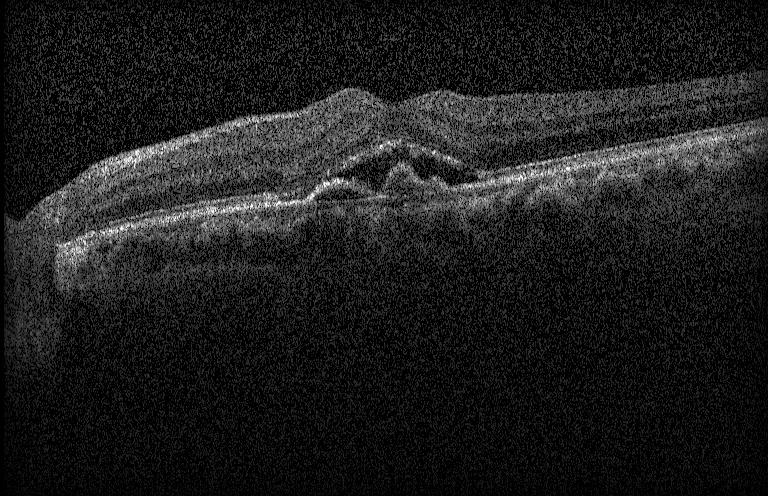 Retinal OCT B-scan
Impression: a choroidal neovascular membrane.